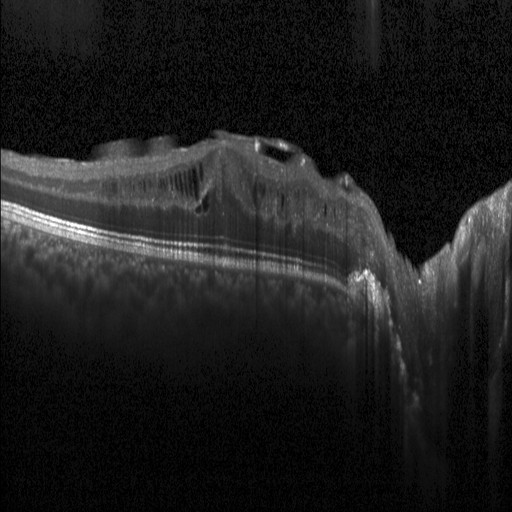 Finding: diabetic macular edema (DME).